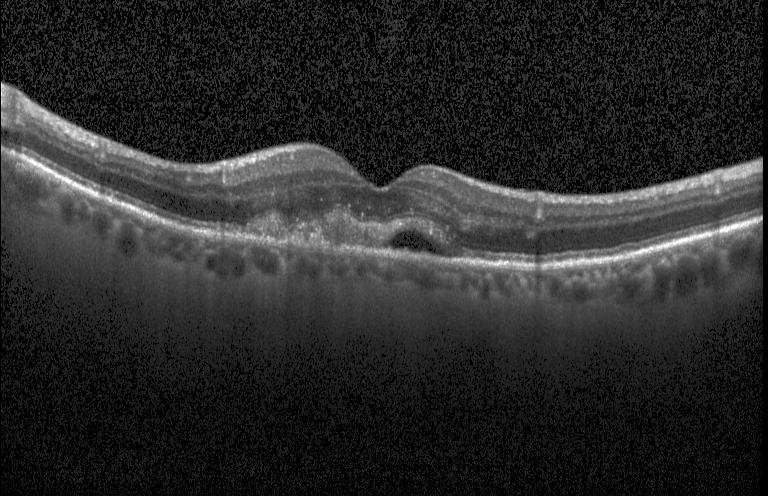

Instrument: Heidelberg Spectralis · spectral-domain optical coherence tomography · through the macula · retinal OCT B-scan — Macular OCT: choroidal neovascularization (CNV).